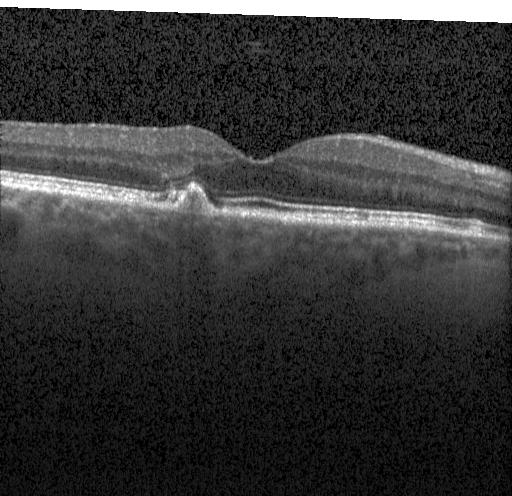

Macular OCT: choroidal neovascularization (CNV).